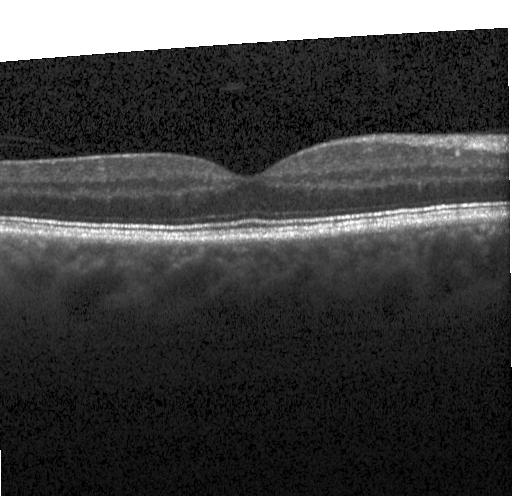 Macular OCT: no evidence of CNV, DME, or drusen.